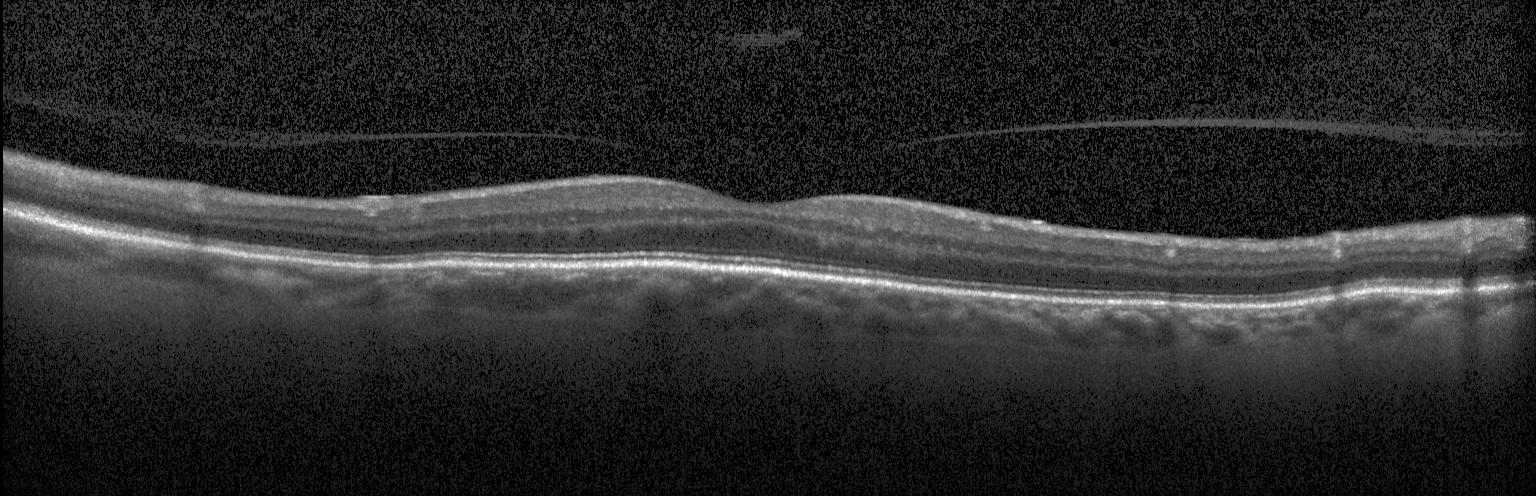 OCT B-scan showing neither choroidal neovascularization, diabetic macular edema, nor drusen.